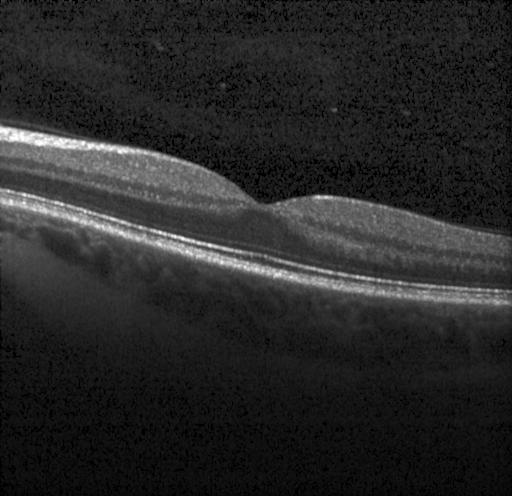
Acquired on a Heidelberg Spectralis; retinal OCT cross-section; centered on the fovea — Diagnosis: no choroidal neovascularization, no diabetic macular edema, and no drusen.